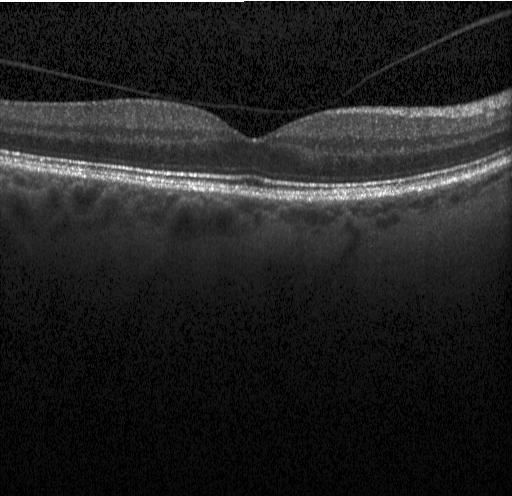
Acquired on a Heidelberg Spectralis · fovea-centered · SD-OCT · retinal OCT B-scan
The scan shows no CNV, DME, or drusen.